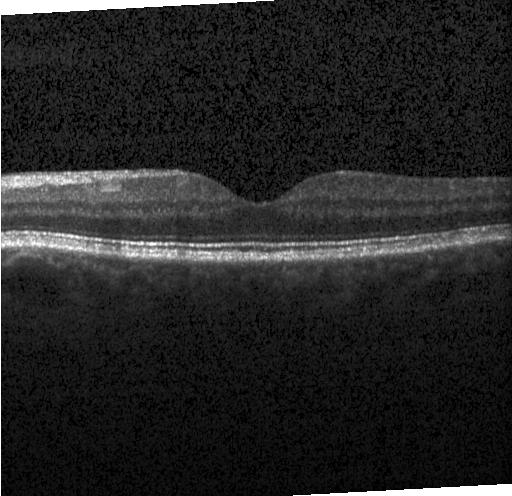 OCT line scan · centered on the fovea · Heidelberg Spectralis OCT system · SD-OCT.
Finding: neither choroidal neovascularization, diabetic macular edema, nor drusen.